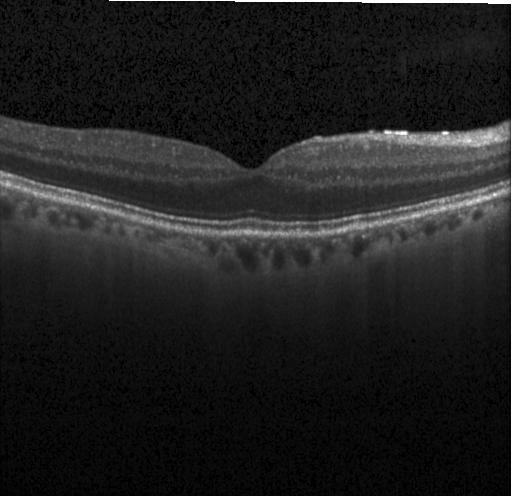

OCT scan showing no choroidal neovascularization, no diabetic macular edema, and no drusen.